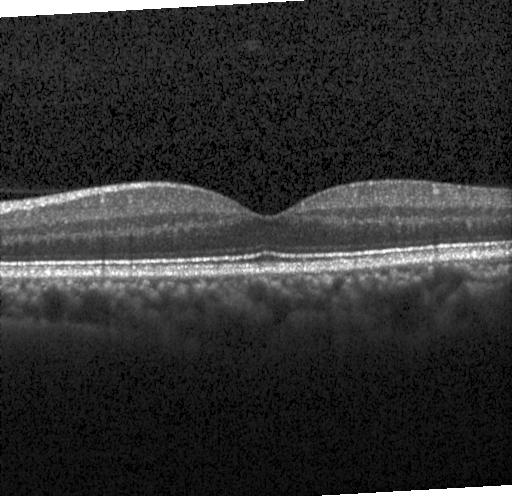

Acquired on a Heidelberg Spectralis · OCT B-scan · SD-OCT · centered on the fovea. Finding: no choroidal neovascularization, no diabetic macular edema, and no drusen.